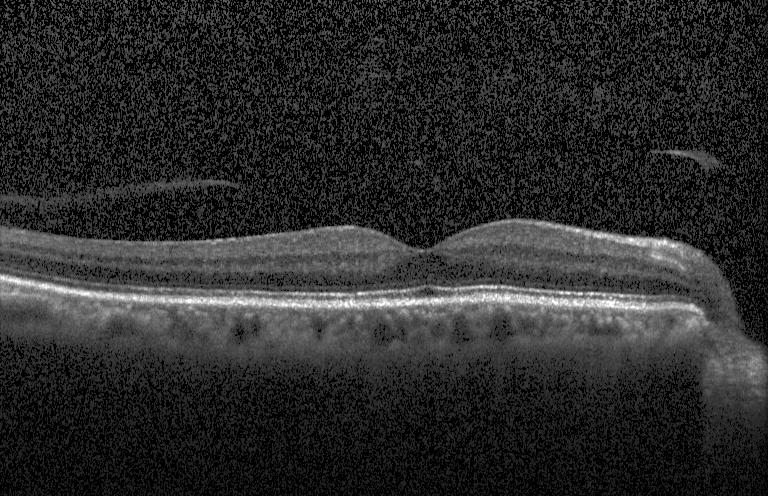 Heidelberg Spectralis OCT system; centered on the fovea; retinal OCT B-scan; spectral-domain optical coherence tomography — Assessment: no choroidal neovascularization, no diabetic macular edema, and no drusen.